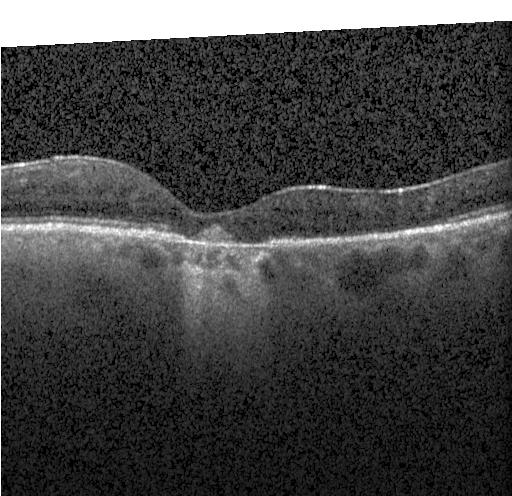
Finding: a choroidal neovascular membrane.